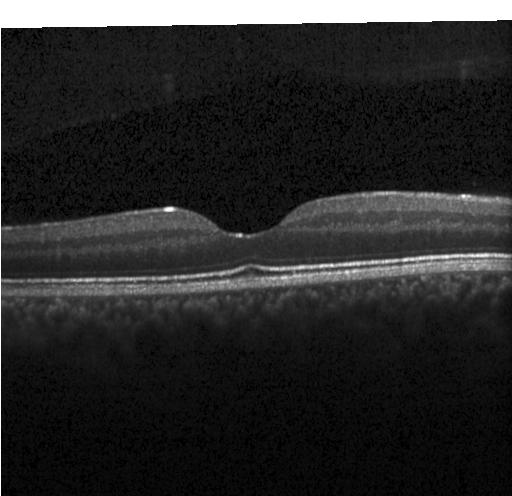
Macular OCT demonstrating no evidence of choroidal neovascularization, diabetic macular edema, or drusen.